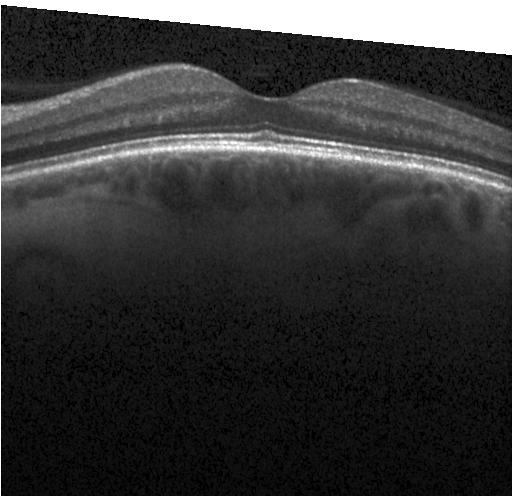

Fovea-centered; OCT line scan; spectral-domain OCT. Finding: no evidence of choroidal neovascularization, diabetic macular edema, or drusen.